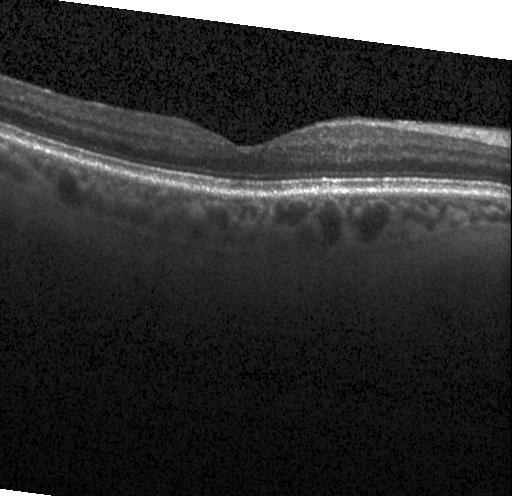

Diagnosis: no choroidal neovascularization, diabetic macular edema, or drusen.